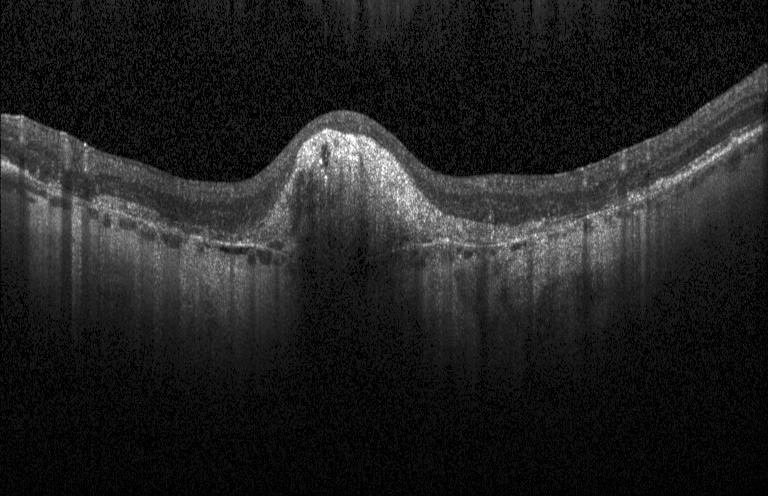

Fovea-centered · acquired on a Heidelberg Spectralis · OCT B-scan · spectral-domain OCT — This B-scan demonstrates CNV.